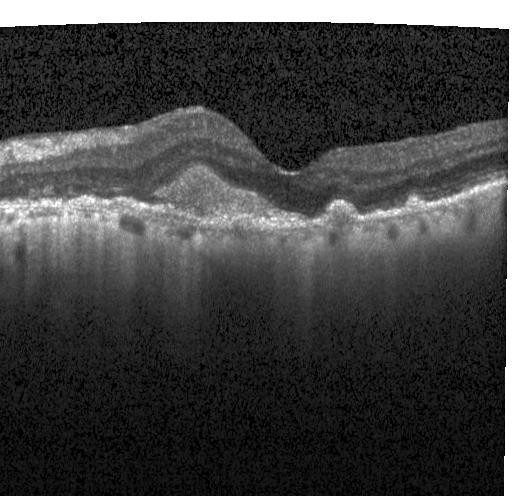 Spectral-domain OCT B-scan: a choroidal neovascular membrane.